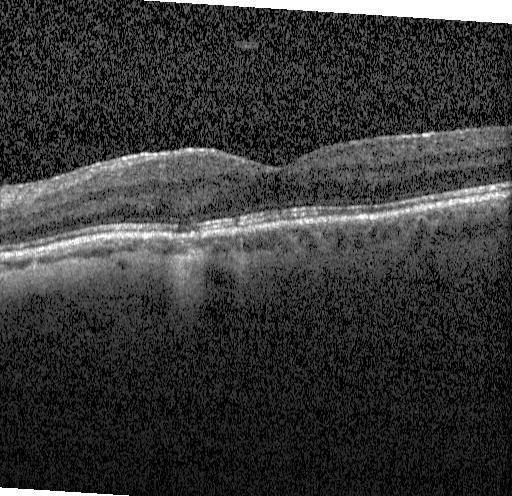
Retinal OCT cross-section showing no choroidal neovascularization, no diabetic macular edema, and no drusen.